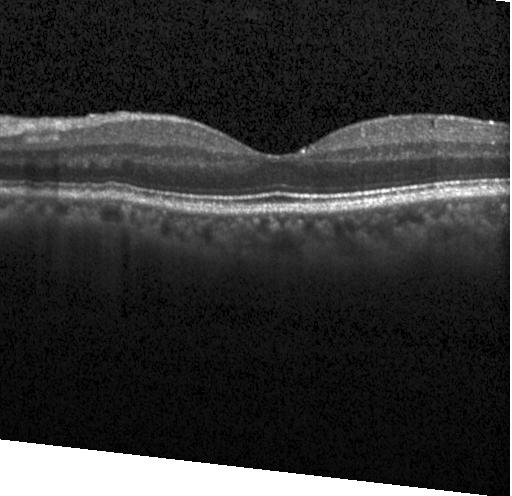 Acquired on a Heidelberg Spectralis, spectral-domain optical coherence tomography, retinal OCT B-scan. Assessment: no choroidal neovascularization, no diabetic macular edema, and no drusen.